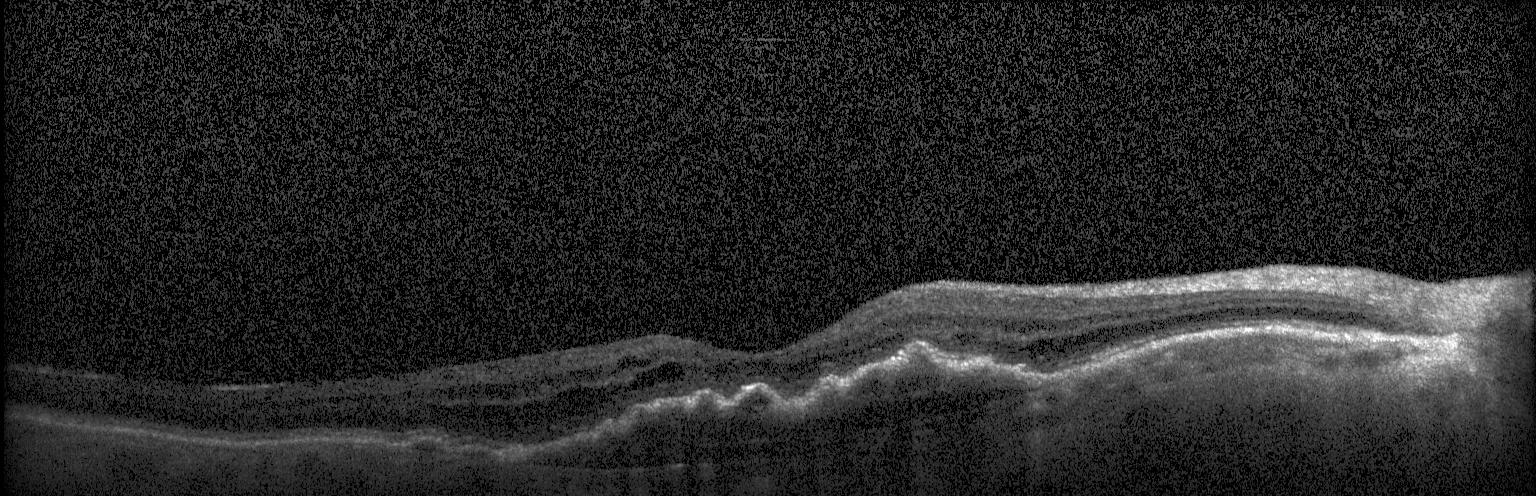

Fovea-centered. Optical coherence tomography scan — This B-scan demonstrates a choroidal neovascular membrane.